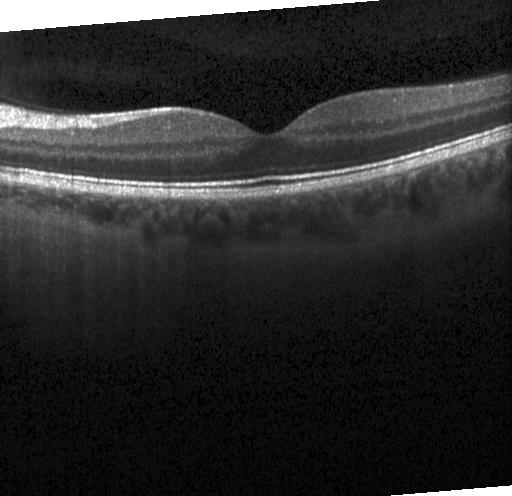

Impression: neither choroidal neovascularization, diabetic macular edema, nor drusen.